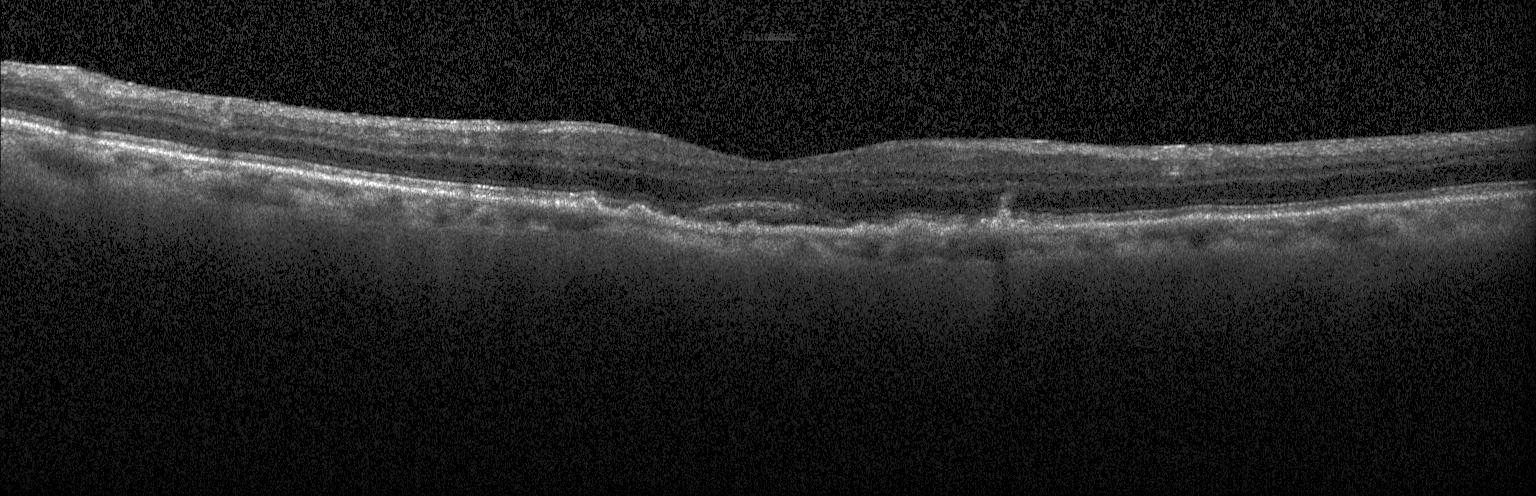 Macular OCT demonstrating choroidal neovascularization (CNV).